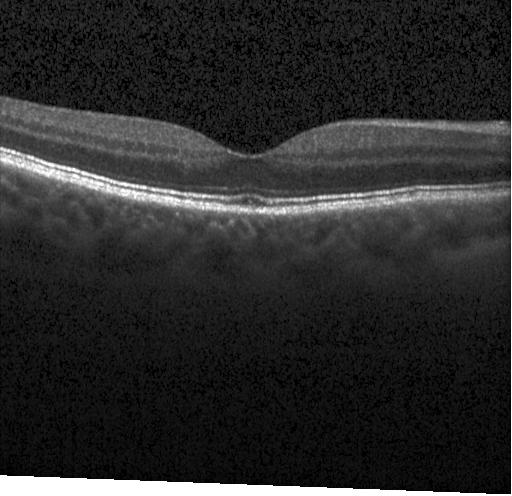

OCT scan showing no evidence of choroidal neovascularization, diabetic macular edema, or drusen.